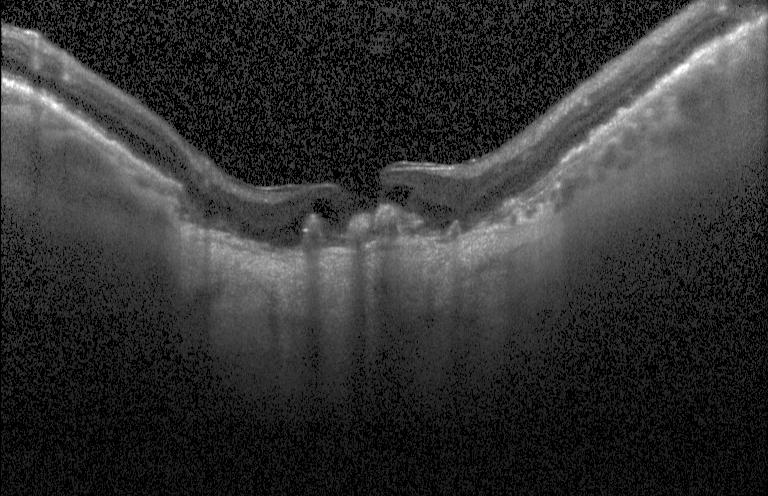

Macular OCT: a choroidal neovascular membrane.